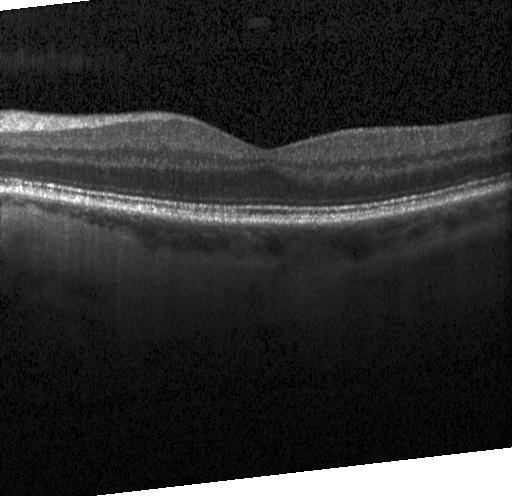

Instrument: Heidelberg Spectralis · optical coherence tomography B-scan · macular scan.
OCT finding: no choroidal neovascularization, no diabetic macular edema, and no drusen.